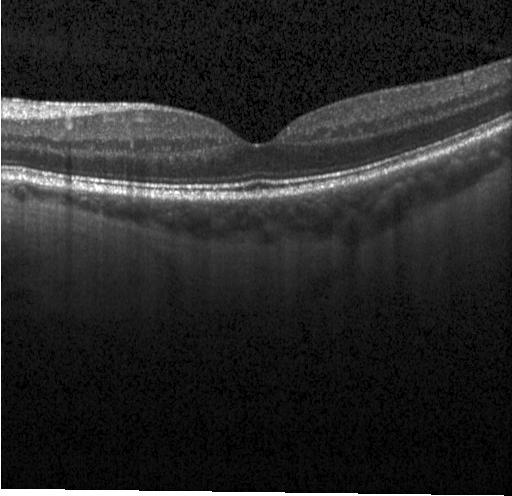

Dx: neither CNV, DME, nor drusen.